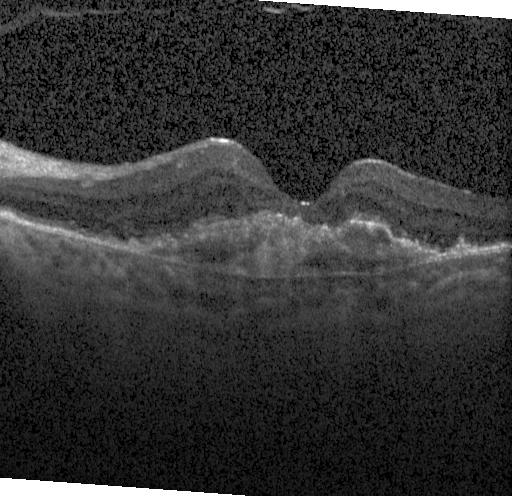 Spectral-domain optical coherence tomography. Retinal OCT B-scan. Macular scan. CNV.